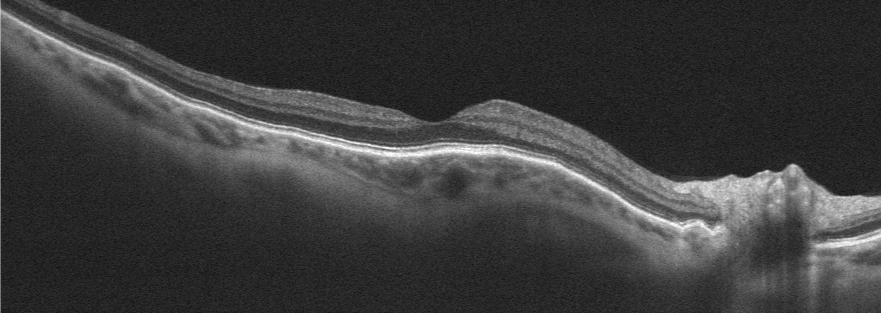
OCT line scan. Macular OCT: absence of AMD, DME, ERM, RAO, RVO, and vitreomacular interface disease.